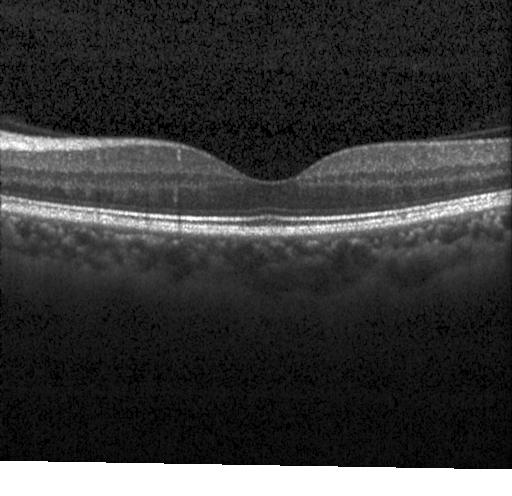
Assessment: no choroidal neovascularization, no diabetic macular edema, and no drusen.